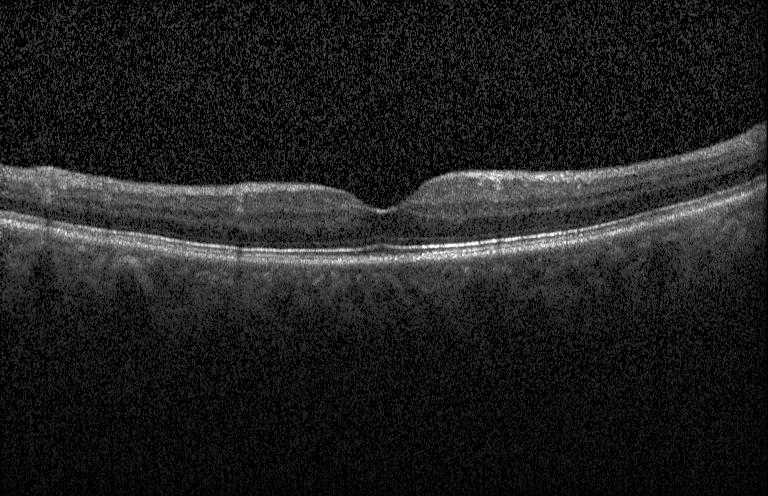
Diagnosis: no evidence of CNV, DME, or drusen.